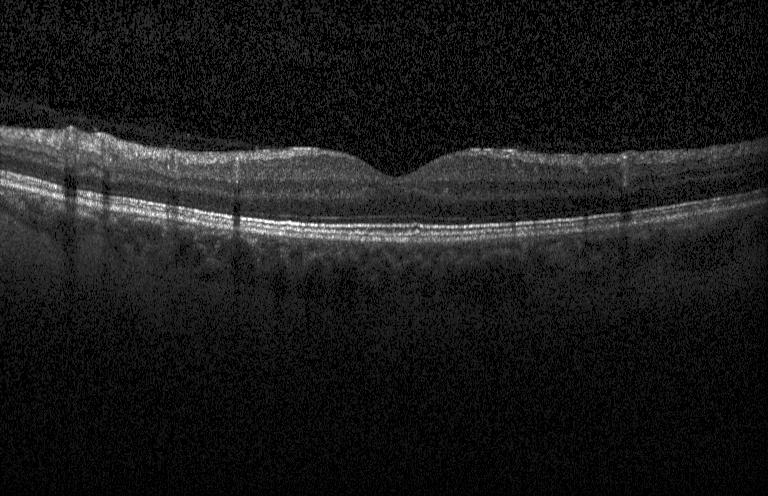 Retinal OCT cross-section. Horizontal scan through the fovea
Dx: no choroidal neovascularization, no diabetic macular edema, and no drusen.